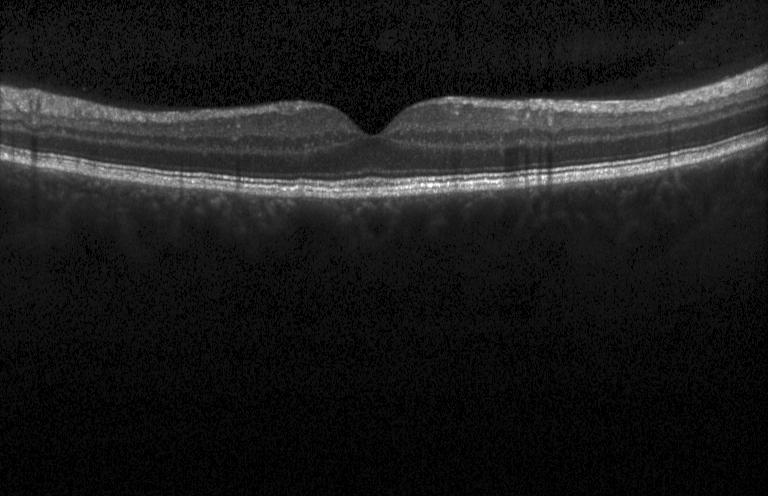 Spectral-domain OCT; optical coherence tomography scan. Dx: no choroidal neovascularization, diabetic macular edema, or drusen.